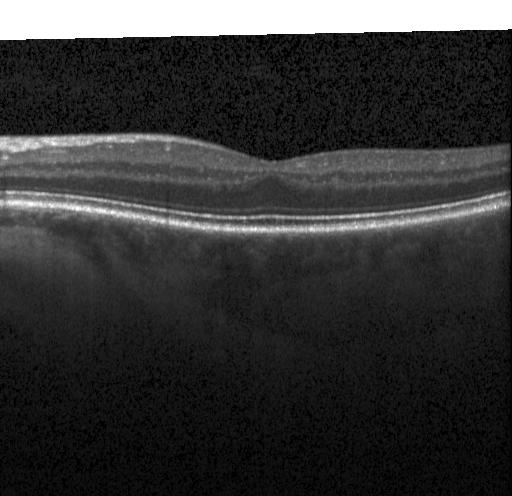

Assessment: no evidence of choroidal neovascularization, diabetic macular edema, or drusen.